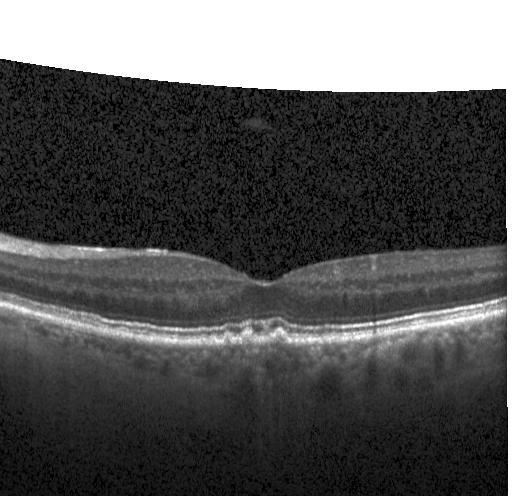
Heidelberg Spectralis OCT system; retinal OCT B-scan
Finding: sub-RPE drusenoid deposits.